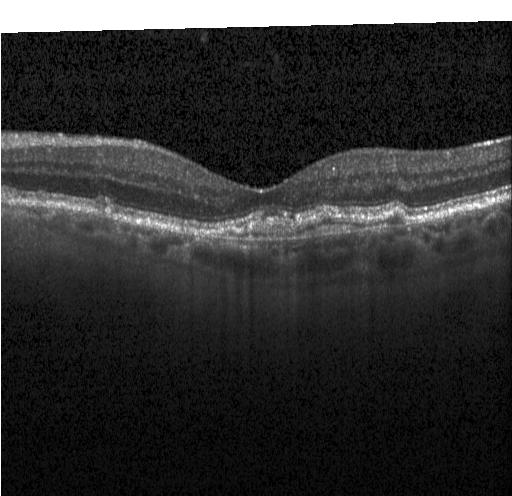

Through the macula, OCT line scan, spectral-domain optical coherence tomography — OCT finding: a choroidal neovascular membrane.